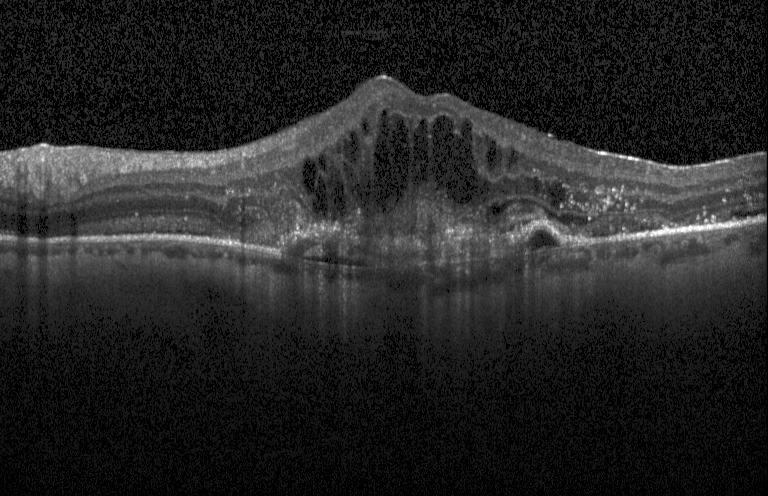

Heidelberg Spectralis; OCT line scan; spectral-domain OCT; through the macula.
This B-scan demonstrates a choroidal neovascular membrane.